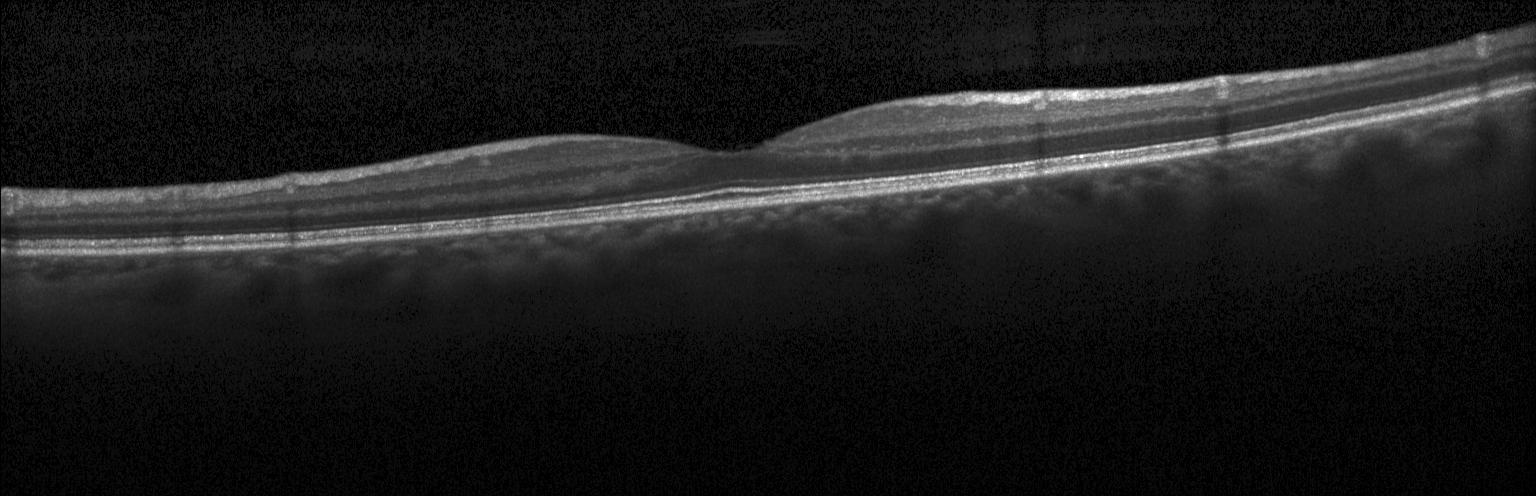

Diagnosis: no evidence of choroidal neovascularization, diabetic macular edema, or drusen.